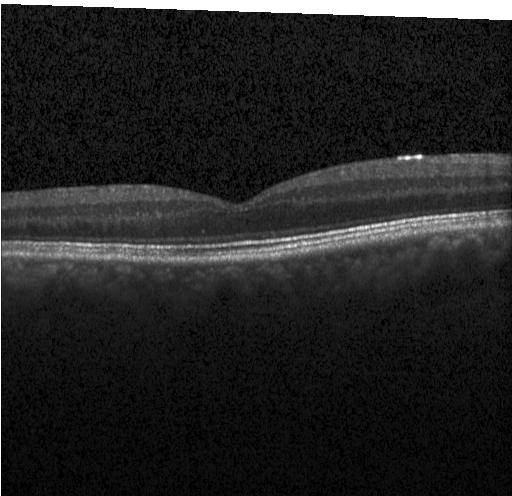
Assessment: neither choroidal neovascularization, diabetic macular edema, nor drusen.